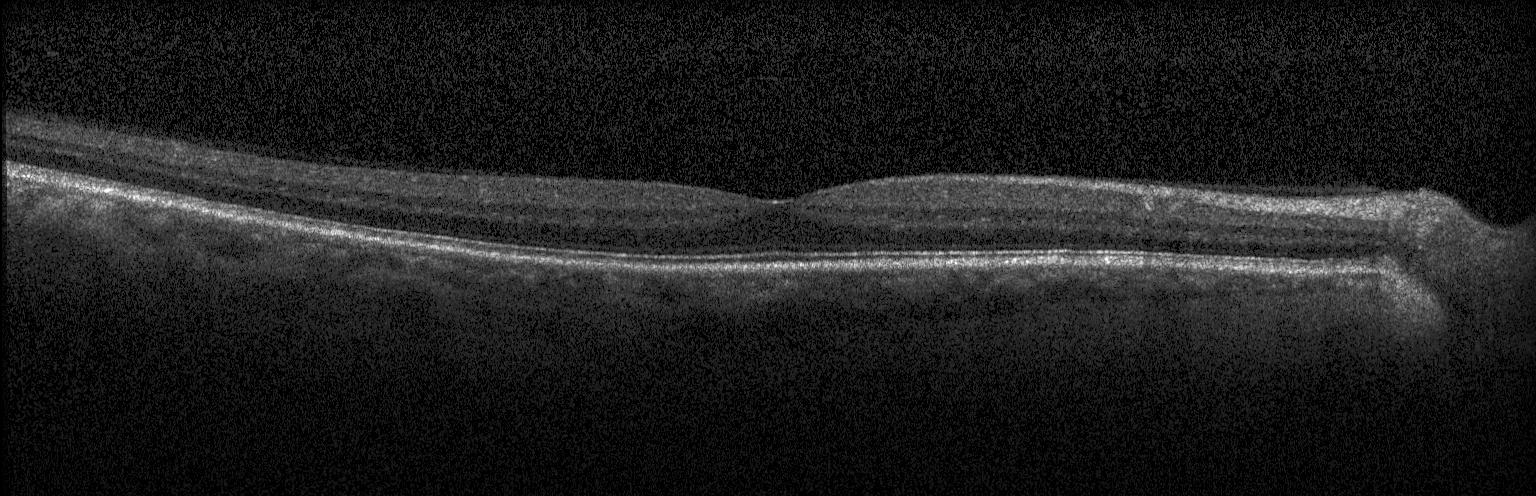 Instrument: Heidelberg Spectralis · retinal OCT B-scan · spectral-domain OCT · horizontal scan through the fovea
Finding: neither choroidal neovascularization, diabetic macular edema, nor drusen.